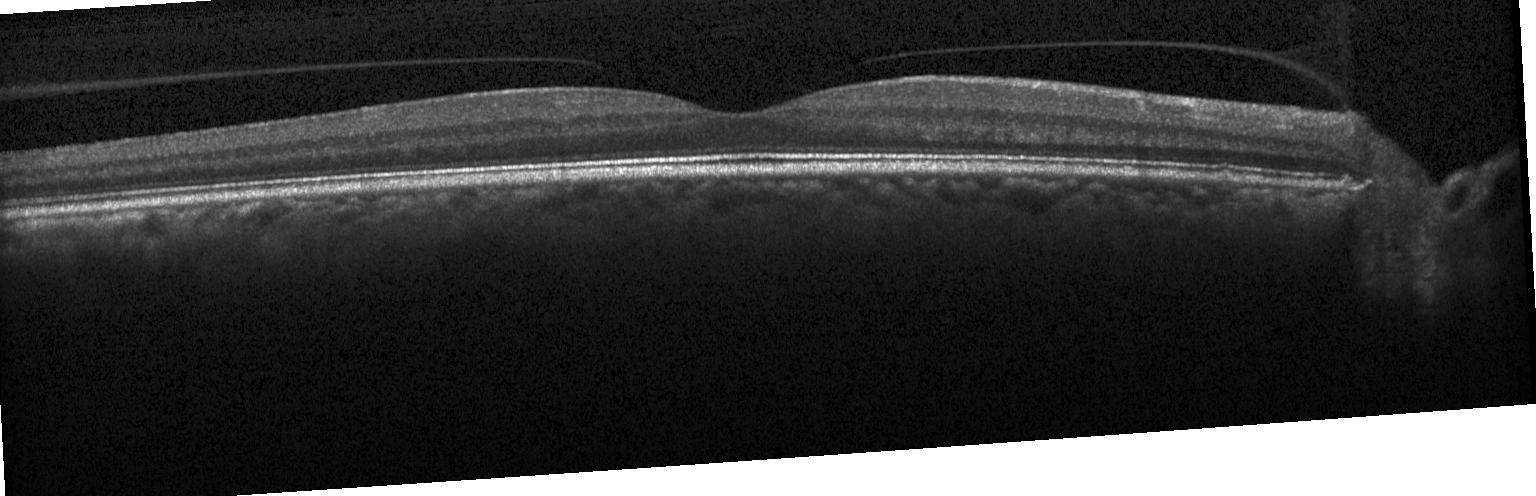

Impression: no evidence of choroidal neovascularization, diabetic macular edema, or drusen.